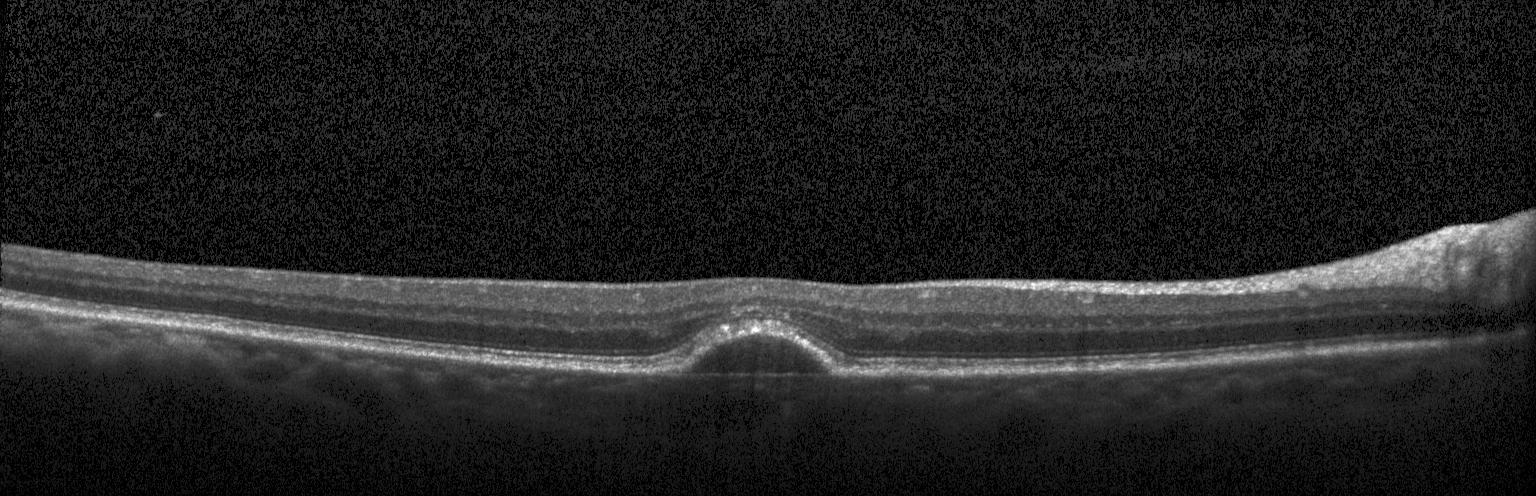

Macular OCT: choroidal neovascularization (CNV).